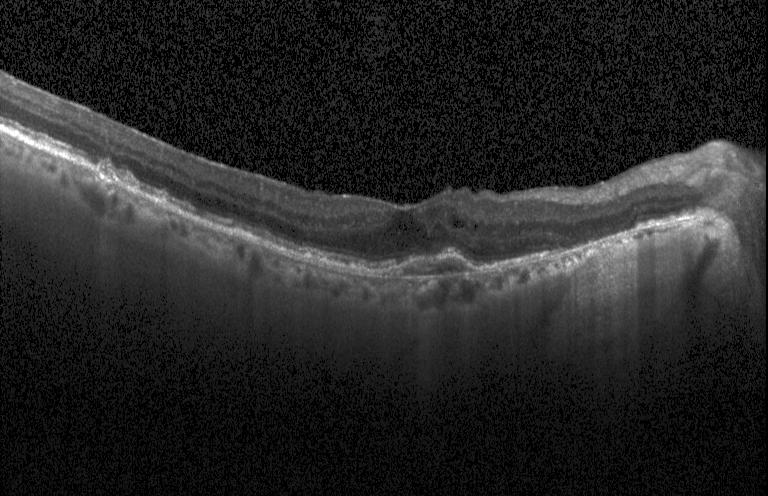
Acquired on a Heidelberg Spectralis · SD-OCT · optical coherence tomography scan · fovea-centered.
Impression: a choroidal neovascular membrane.